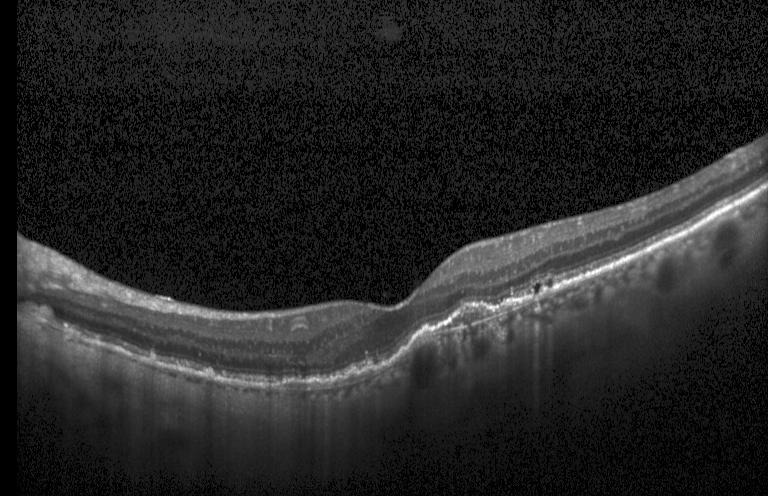

Retinal OCT B-scan · Heidelberg Spectralis · spectral-domain OCT · through the macula. This B-scan demonstrates a choroidal neovascular membrane.